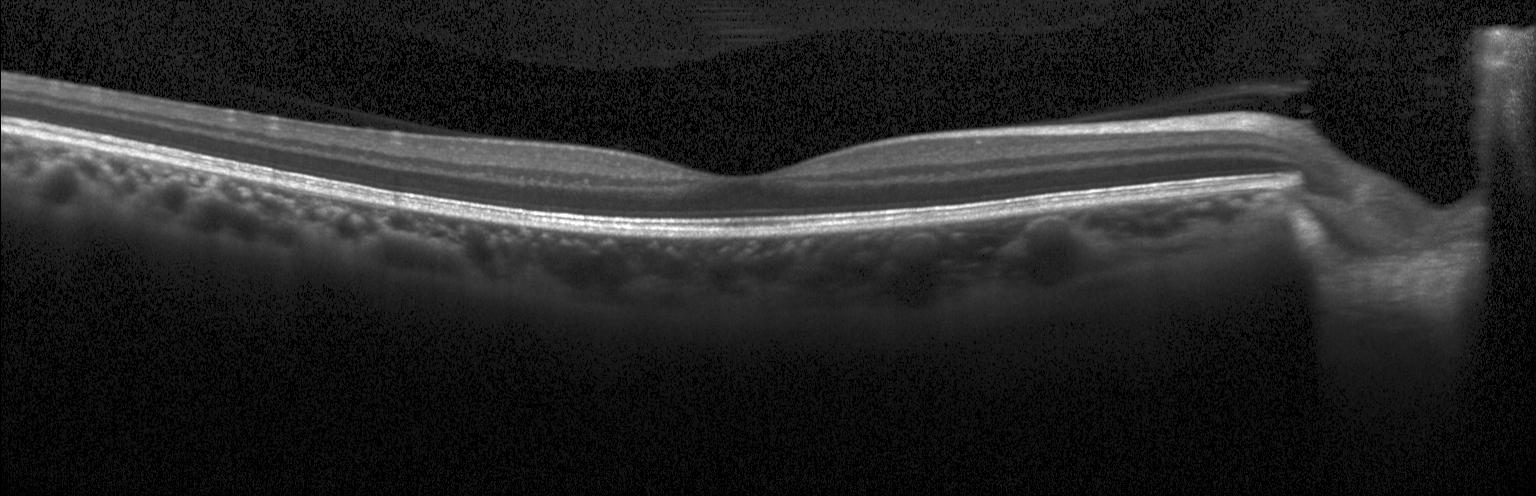

OCT line scan · Heidelberg Spectralis · SD-OCT — Impression: no evidence of choroidal neovascularization, diabetic macular edema, or drusen.